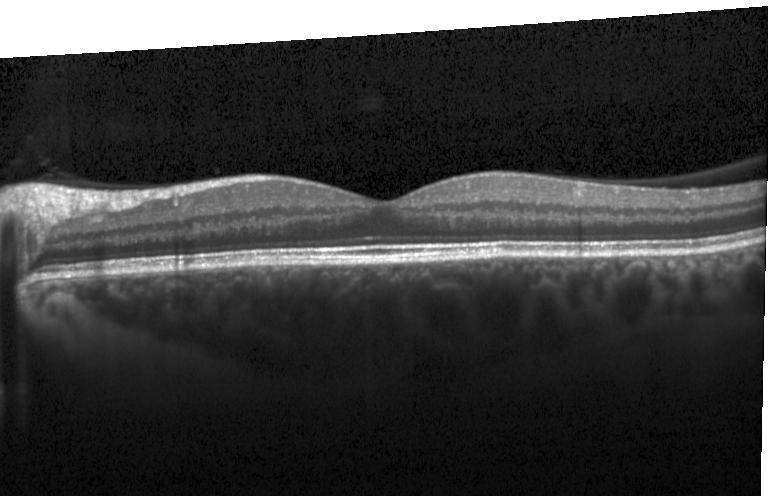 Optical coherence tomography scan. Diagnosis: neither choroidal neovascularization, diabetic macular edema, nor drusen.